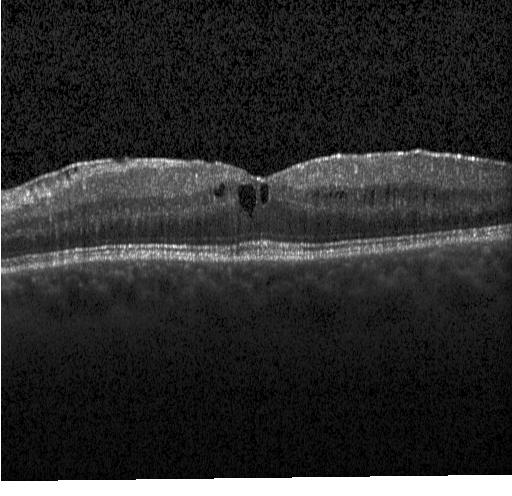 OCT finding: DME.